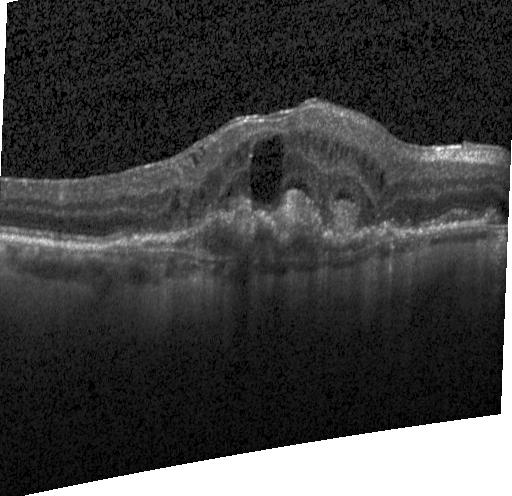

Spectral-domain OCT B-scan: a choroidal neovascular membrane.